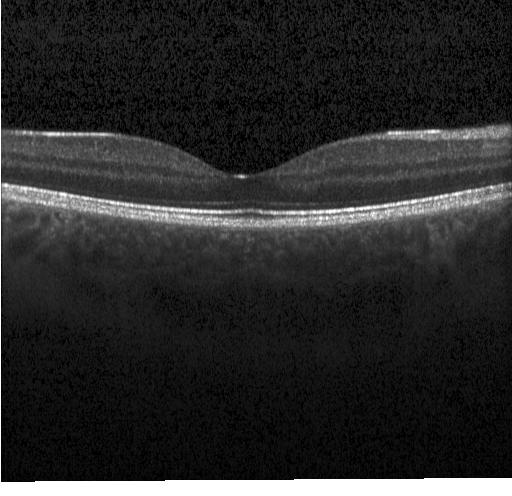
Through the macula · SD-OCT · optical coherence tomography scan · acquired on a Heidelberg Spectralis
Dx: no choroidal neovascularization, diabetic macular edema, or drusen.